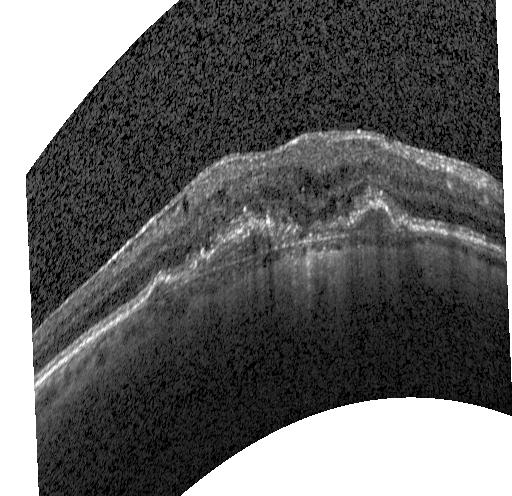
OCT B-scan.
Macular OCT: CNV.